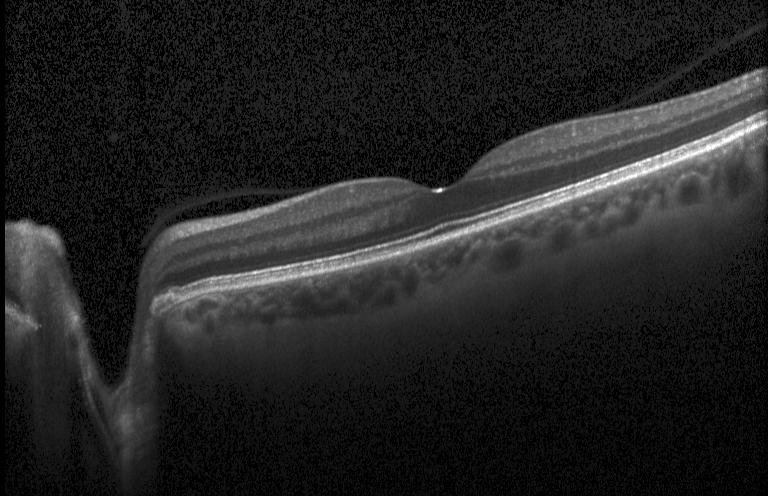 OCT line scan, spectral-domain OCT, fovea-centered, Heidelberg Spectralis.
Finding: neither choroidal neovascularization, diabetic macular edema, nor drusen.